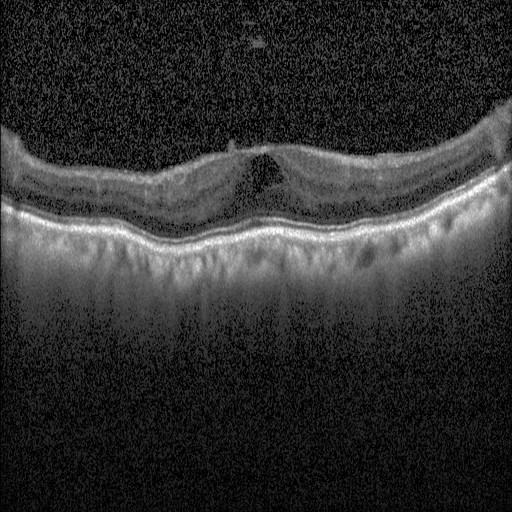

Optical coherence tomography scan. Dx: diabetic macular edema.